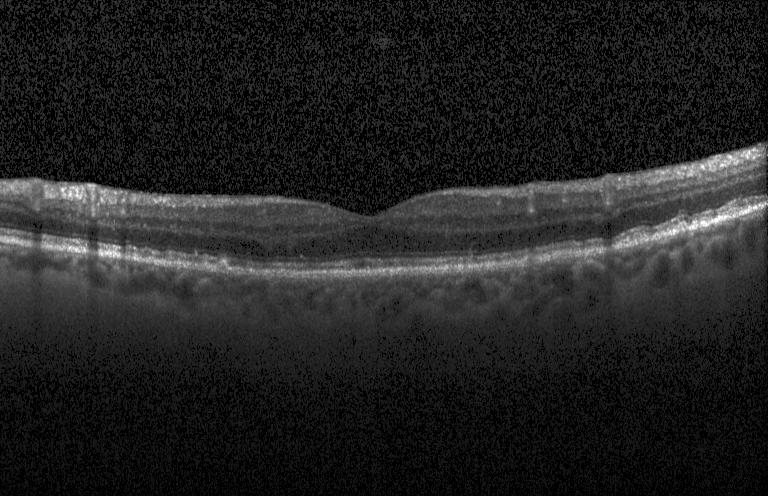
Impression: drusen.